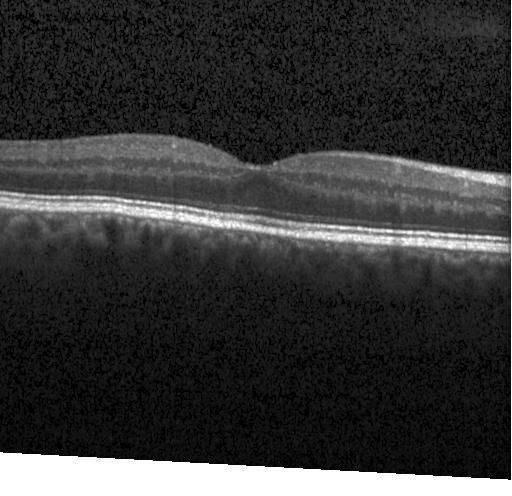

Centered on the fovea. Retinal OCT cross-section — Impression: neither CNV, DME, nor drusen.